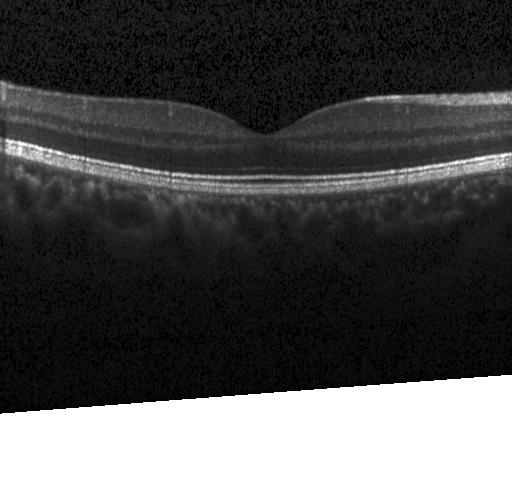 OCT B-scan, spectral-domain optical coherence tomography, centered on the fovea, Heidelberg Spectralis OCT system
Impression: no CNV, no DME, and no drusen.